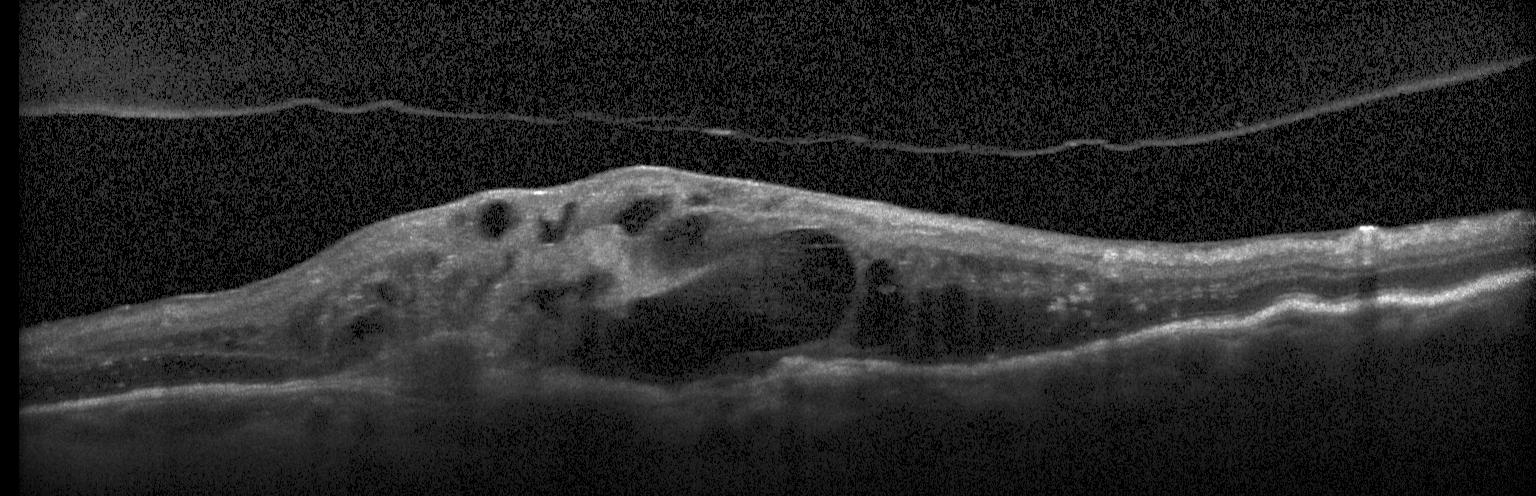

Spectral-domain OCT. Optical coherence tomography B-scan. Macular scan. Acquired on a Heidelberg Spectralis
Impression: a choroidal neovascular membrane.